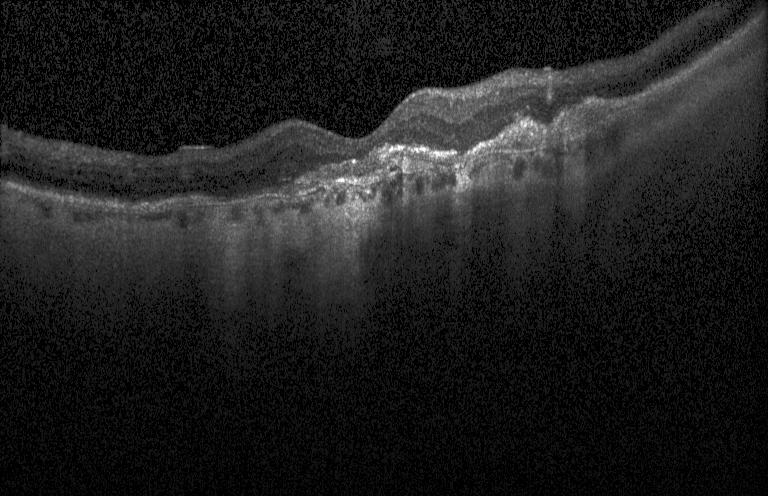

OCT scan showing choroidal neovascularization (CNV).